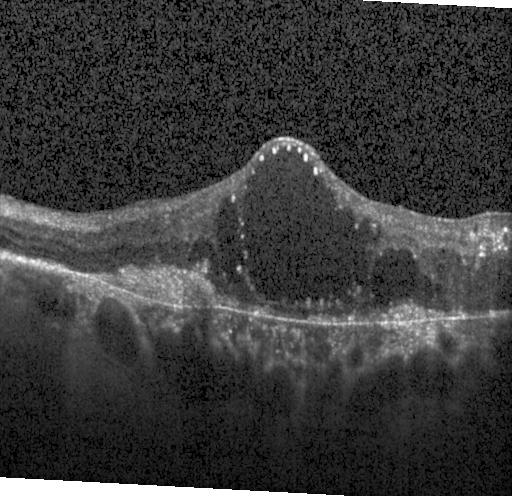 The scan shows choroidal neovascularization (CNV).